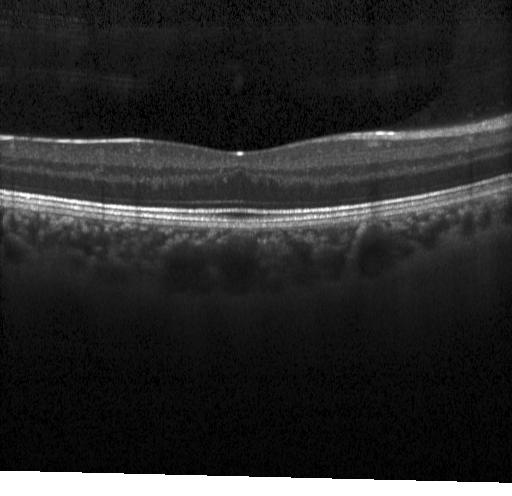
Heidelberg Spectralis. Retinal OCT B-scan. Fovea-centered. Spectral-domain OCT
Impression: no choroidal neovascularization, diabetic macular edema, or drusen.